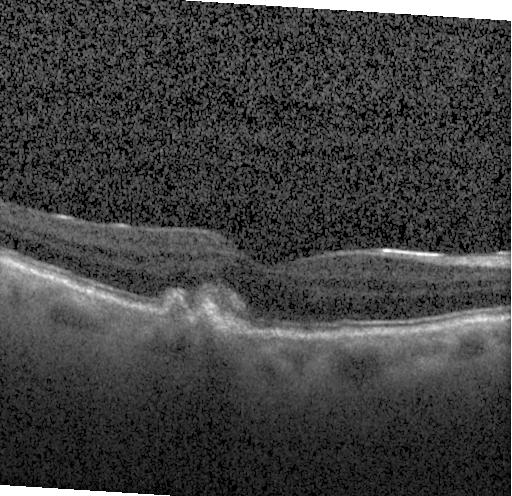

OCT line scan. Macular scan — This B-scan demonstrates CNV.